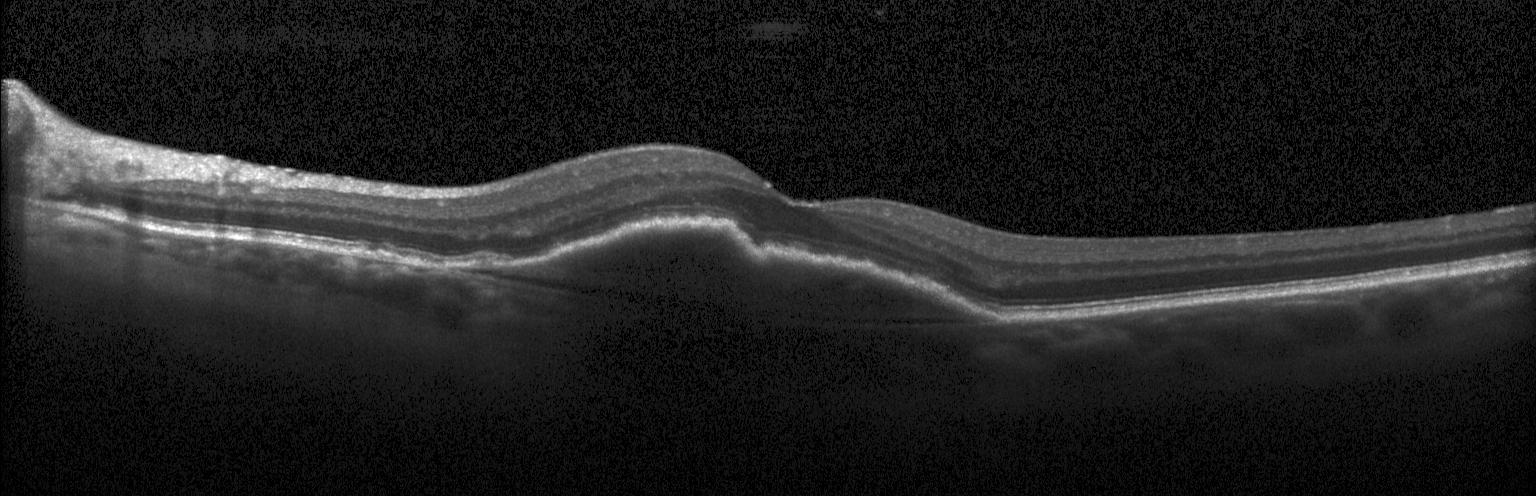
Choroidal neovascularization.